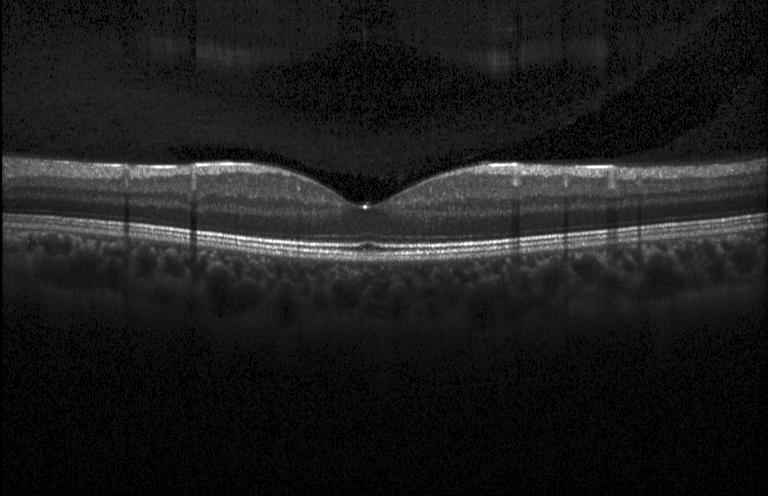

Retinal OCT cross-section showing no choroidal neovascularization, no diabetic macular edema, and no drusen.